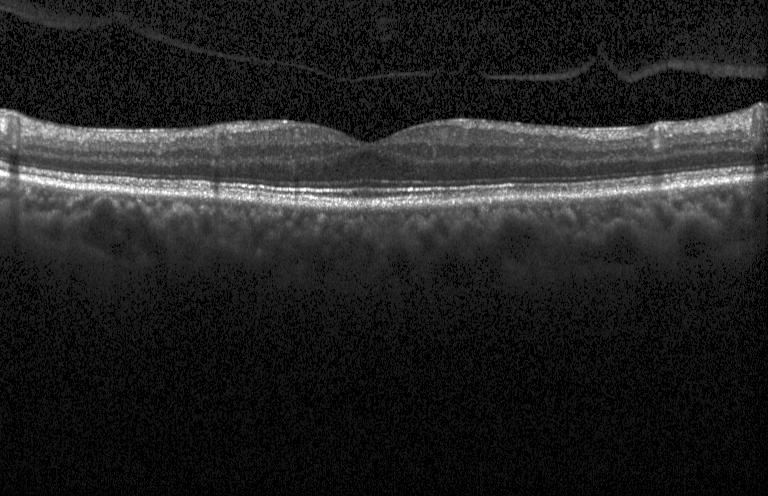 Centered on the fovea, Heidelberg Spectralis OCT system, retinal OCT cross-section, spectral-domain optical coherence tomography
This B-scan demonstrates neither choroidal neovascularization, diabetic macular edema, nor drusen.